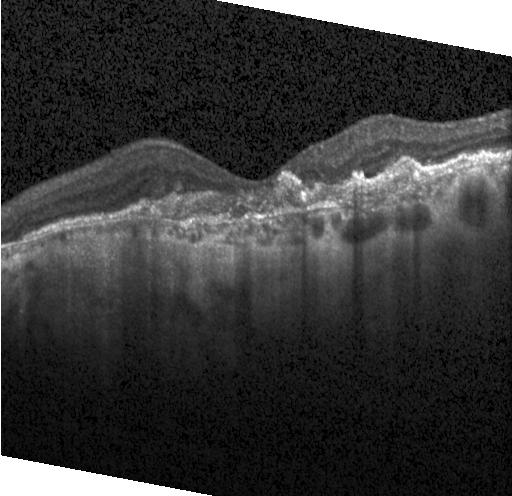 Fovea-centered. OCT B-scan.
Finding: choroidal neovascularization (CNV).